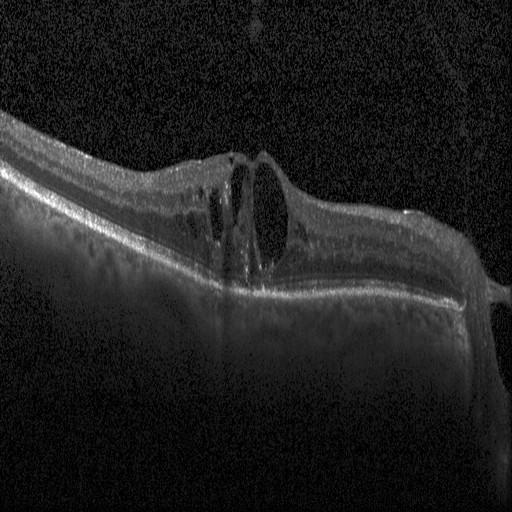

Acquired on a Heidelberg Spectralis; optical coherence tomography B-scan
Finding: diabetic macular edema.